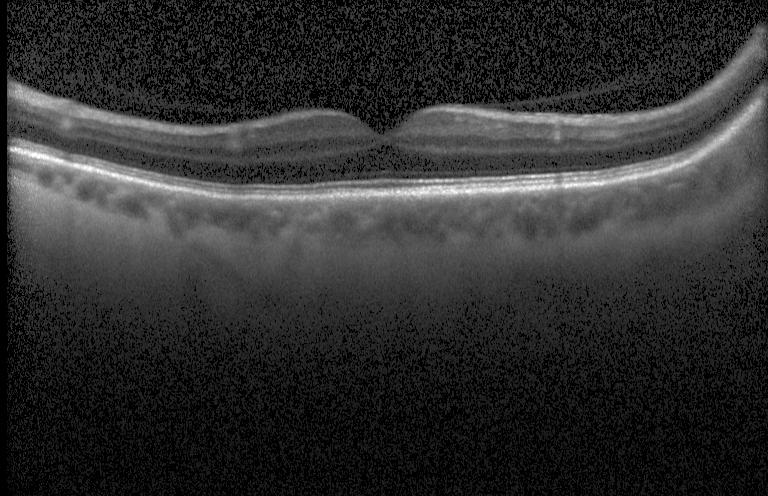
Diagnosis: no CNV, DME, or drusen.